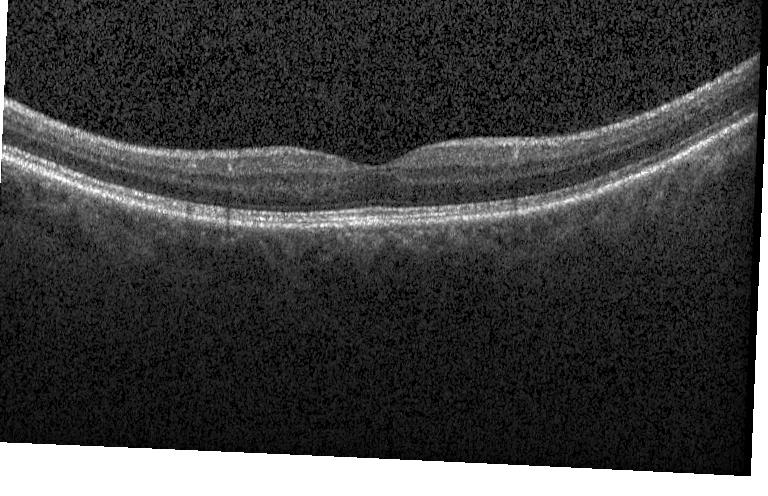 SD-OCT · retinal OCT cross-section · fovea-centered · instrument: Heidelberg Spectralis. Impression: no evidence of choroidal neovascularization, diabetic macular edema, or drusen.